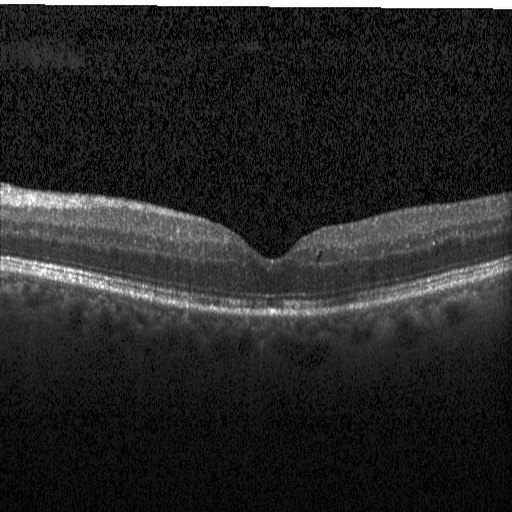 Optical coherence tomography scan
Impression: diabetic macular edema (DME).